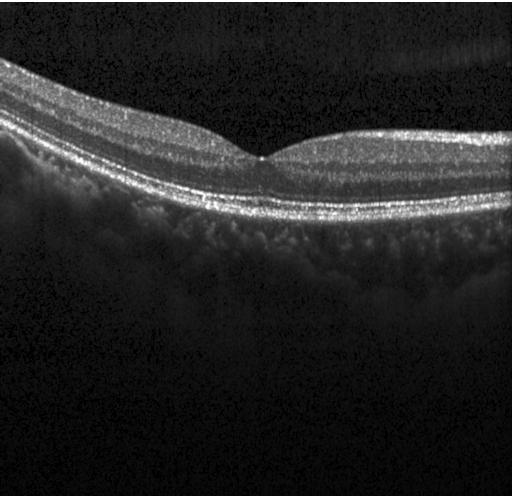 OCT line scan; spectral-domain optical coherence tomography. Finding: no evidence of CNV, DME, or drusen.